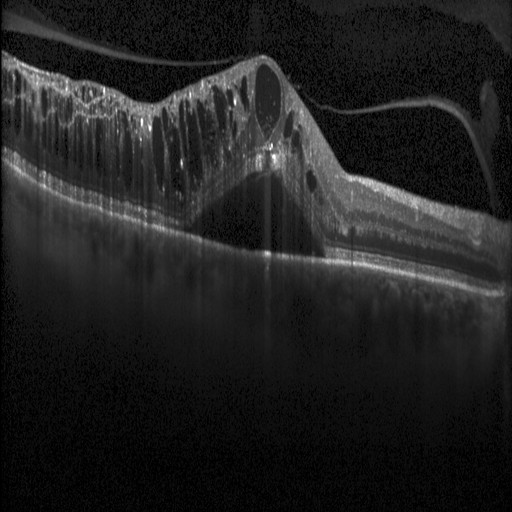

OCT finding: diabetic macular edema.